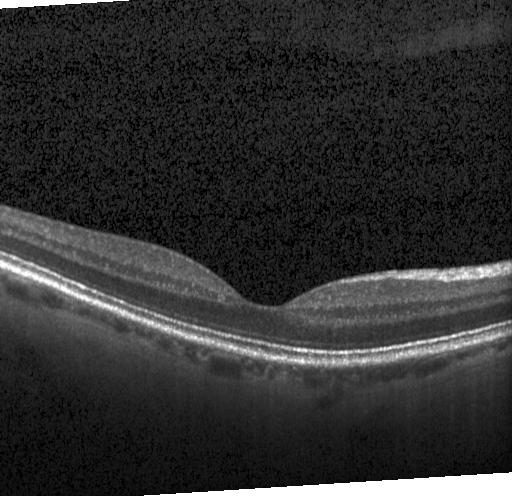

Horizontal scan through the fovea · Heidelberg Spectralis OCT system · SD-OCT · optical coherence tomography B-scan — Macular OCT: no choroidal neovascularization, diabetic macular edema, or drusen.